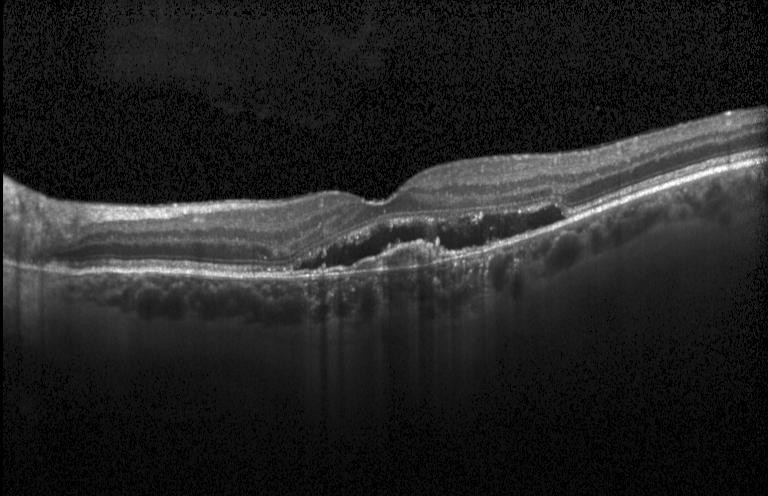
Fovea-centered; OCT line scan; SD-OCT; instrument: Heidelberg Spectralis.
Assessment: choroidal neovascularization.